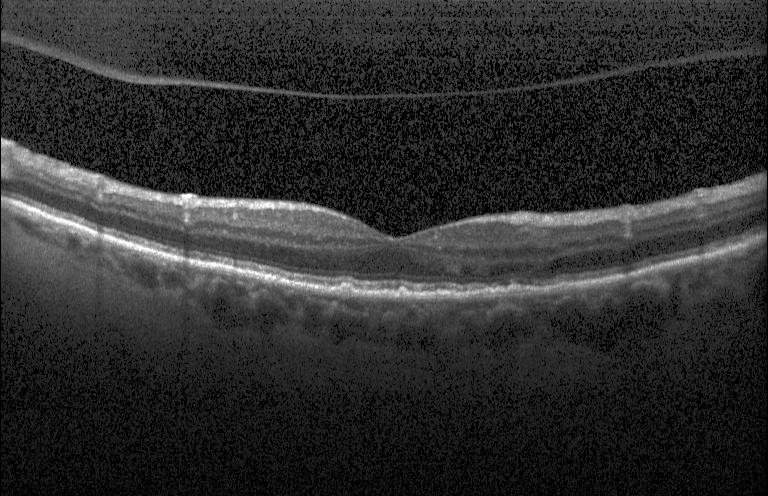 Retinal OCT cross-section · SD-OCT · acquired on a Heidelberg Spectralis — Macular OCT: drusen.